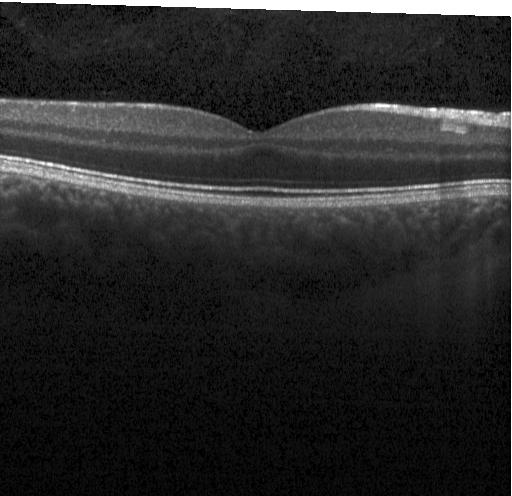

Diagnosis: no evidence of CNV, DME, or drusen.